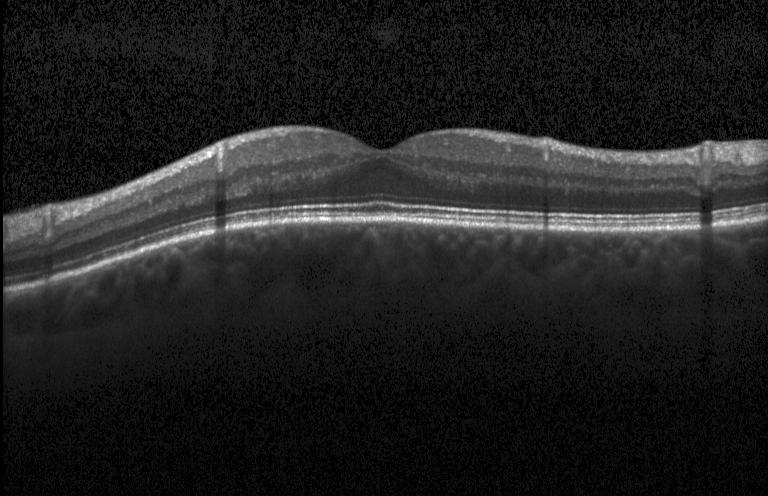

Retinal OCT B-scan, acquired on a Heidelberg Spectralis. Impression: no choroidal neovascularization, no diabetic macular edema, and no drusen.